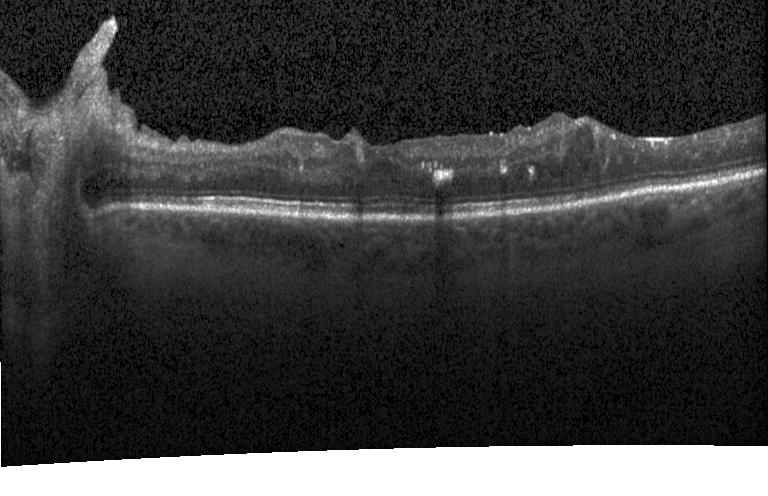 Spectral-domain optical coherence tomography. Optical coherence tomography B-scan. Diabetic macular edema.